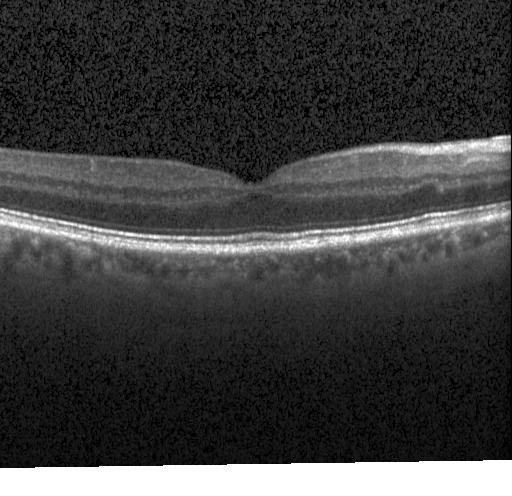

Acquired on a Heidelberg Spectralis · retinal OCT cross-section · centered on the fovea.
Dx: no CNV, DME, or drusen.